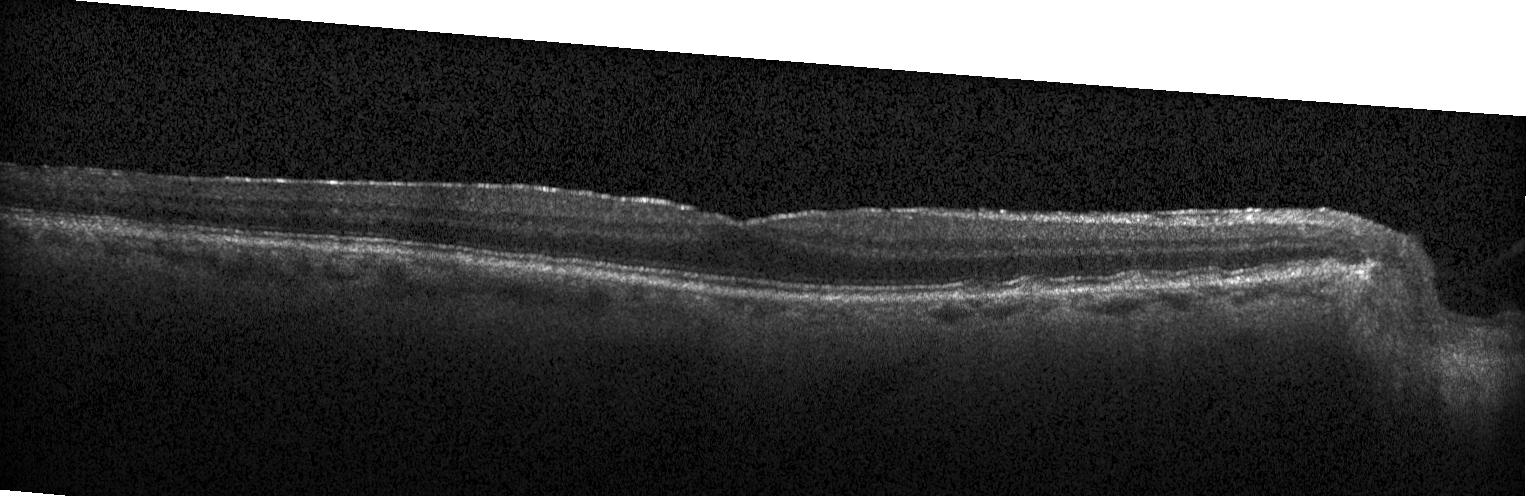
OCT B-scan. Heidelberg Spectralis. Through the macula. SD-OCT.
OCT finding: multiple drusen.